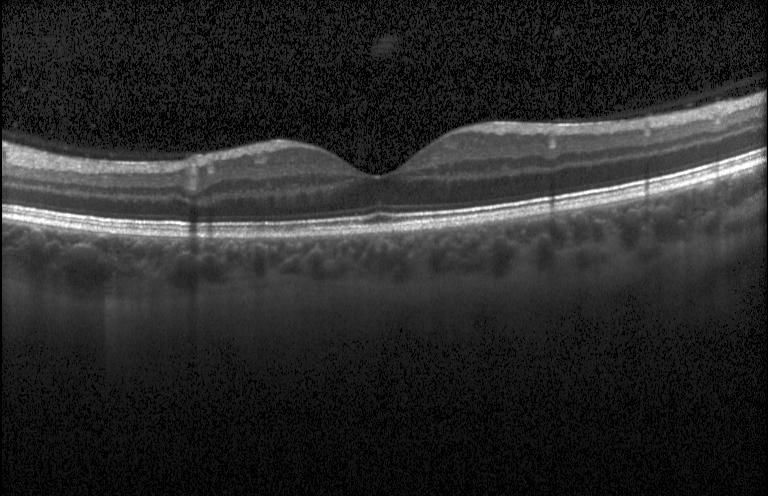 Spectral-domain OCT. Optical coherence tomography scan. Finding: no evidence of choroidal neovascularization, diabetic macular edema, or drusen.